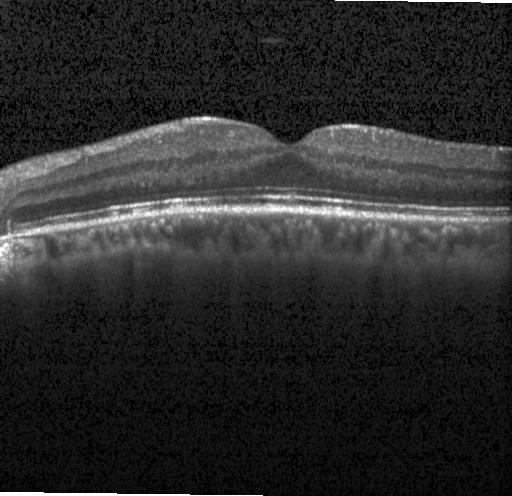 Finding: no choroidal neovascularization, no diabetic macular edema, and no drusen.